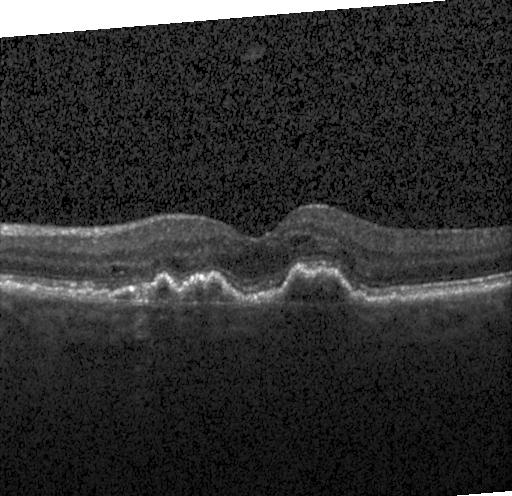

Retinal OCT B-scan, through the macula, spectral-domain optical coherence tomography, Heidelberg Spectralis OCT system.
Finding: choroidal neovascularization (CNV).